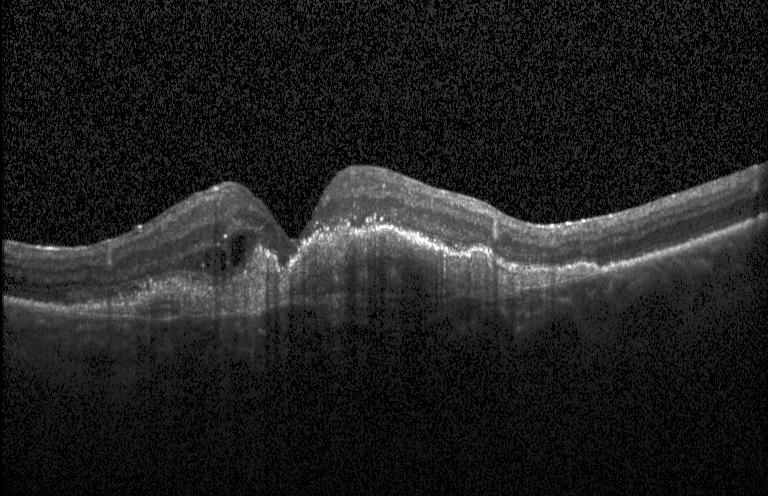 Macular scan; retinal OCT B-scan; acquired on a Heidelberg Spectralis
Diagnosis: a choroidal neovascular membrane.